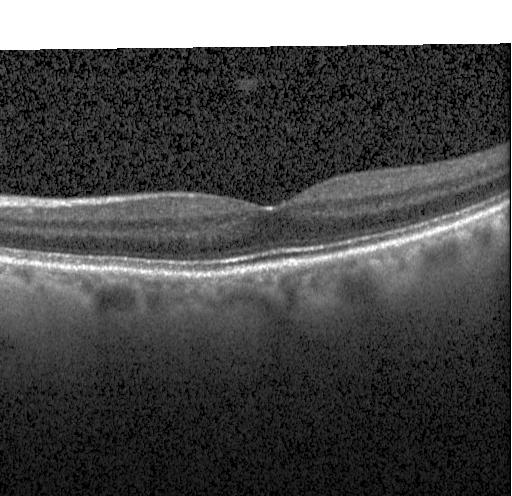

Diagnosis: no choroidal neovascularization, no diabetic macular edema, and no drusen.